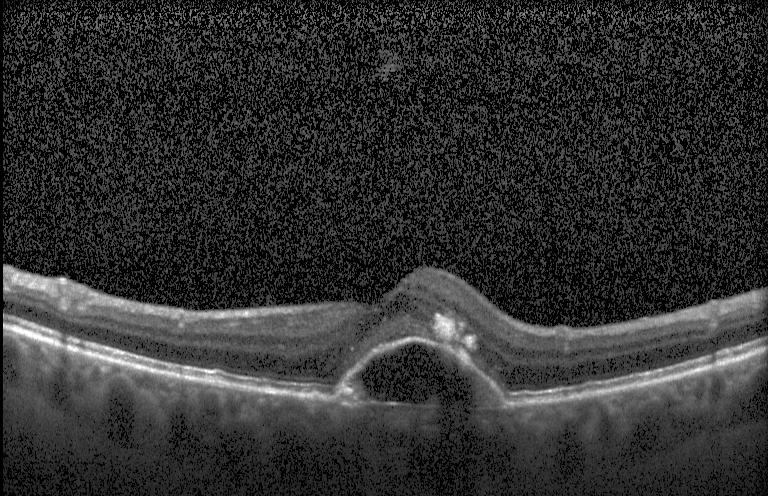 Instrument: Heidelberg Spectralis · spectral-domain optical coherence tomography · fovea-centered · OCT line scan. This B-scan demonstrates CNV.